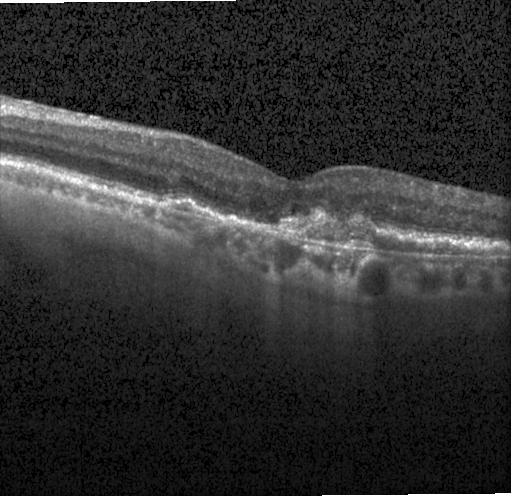 Optical coherence tomography B-scan; instrument: Heidelberg Spectralis
Finding: choroidal neovascularization.